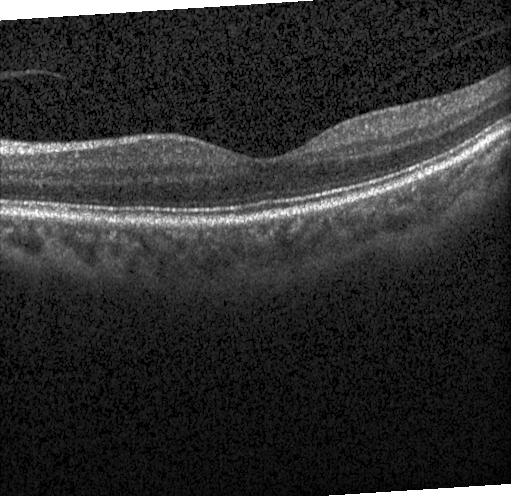

Centered on the fovea, OCT B-scan. Diagnosis: no choroidal neovascularization, diabetic macular edema, or drusen.